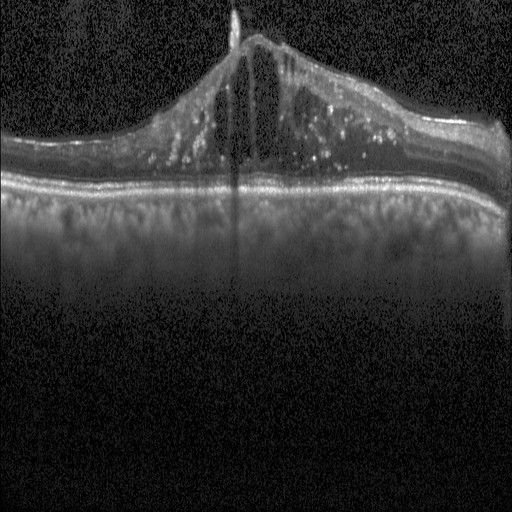 Centered on the fovea. SD-OCT. Acquired on a Heidelberg Spectralis. Optical coherence tomography scan.
Diabetic macular edema.